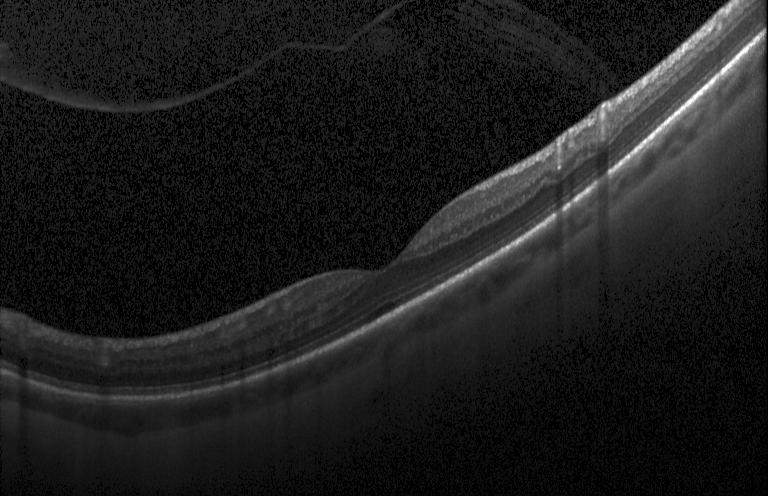

Spectral-domain OCT, fovea-centered, Heidelberg Spectralis OCT system, optical coherence tomography scan — Dx: neither choroidal neovascularization, diabetic macular edema, nor drusen.